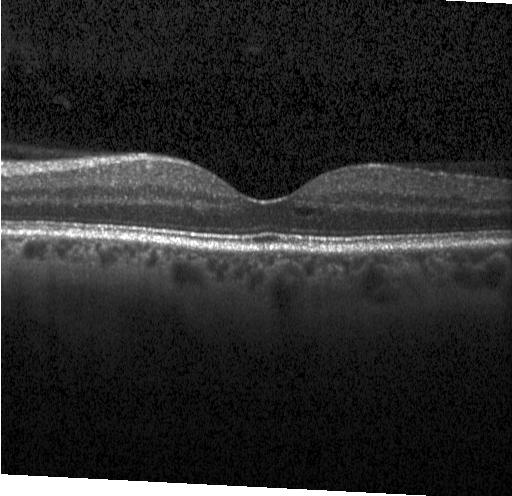 Macular scan; OCT line scan. Diagnosis: neither choroidal neovascularization, diabetic macular edema, nor drusen.